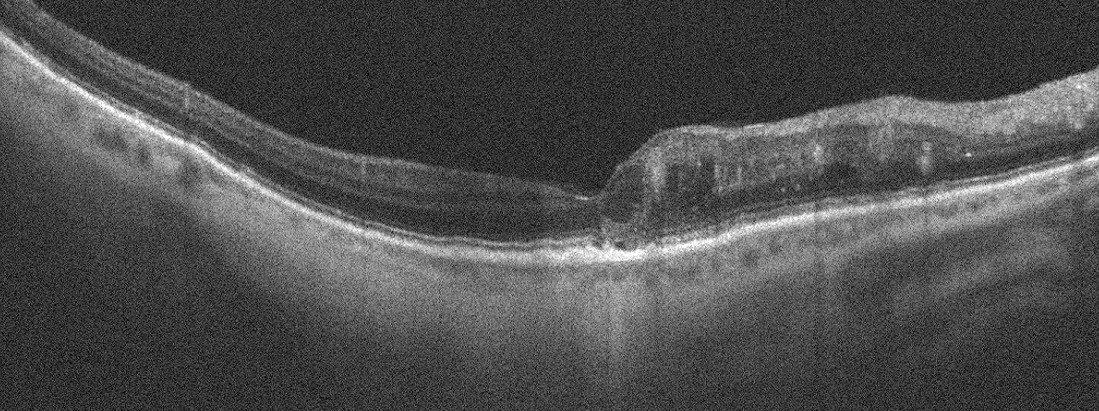
Retinal OCT cross-section — This B-scan demonstrates RVO.